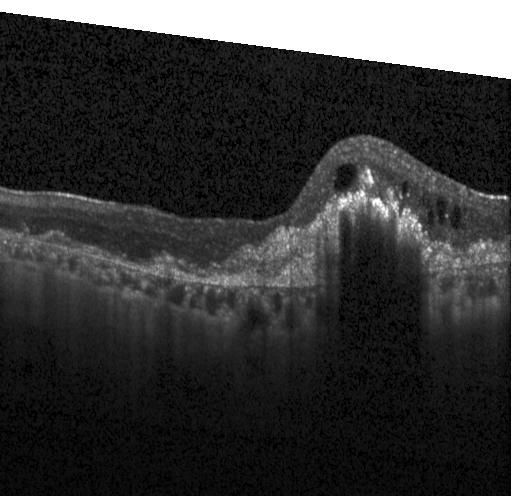

Spectral-domain OCT, fovea-centered, OCT B-scan — Impression: a choroidal neovascular membrane.